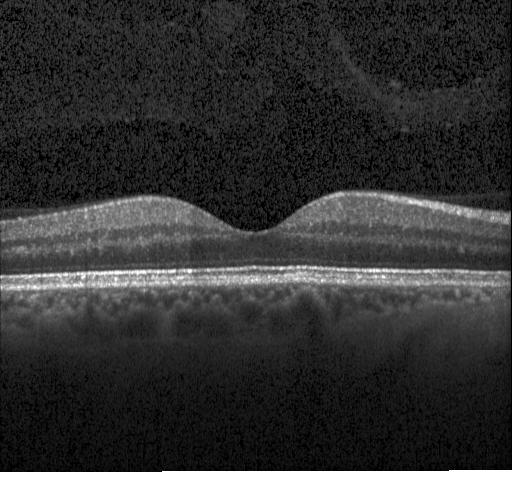

Macular OCT demonstrating no evidence of choroidal neovascularization, diabetic macular edema, or drusen.